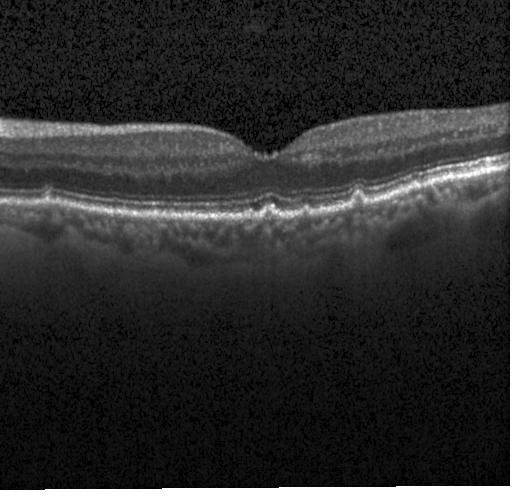 Retinal OCT cross-section, spectral-domain OCT, through the macula — This B-scan demonstrates multiple drusen.